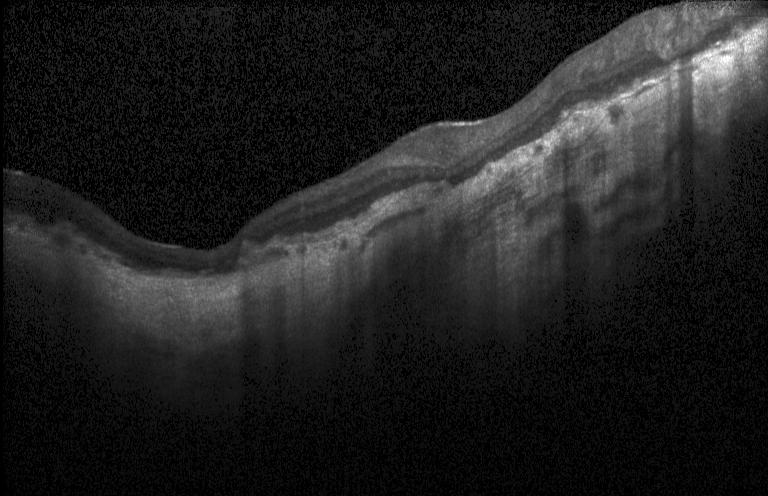 OCT line scan; spectral-domain OCT; acquired on a Heidelberg Spectralis; macular scan.
Impression: a choroidal neovascular membrane.